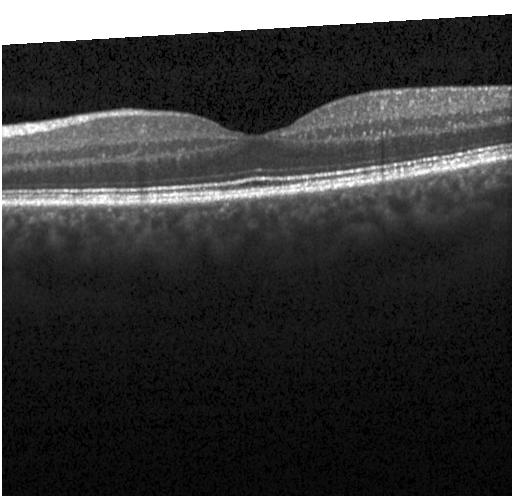

Heidelberg Spectralis · optical coherence tomography scan
Finding: neither CNV, DME, nor drusen.